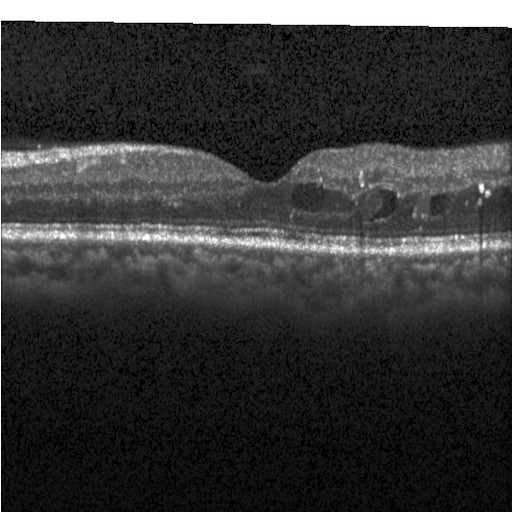

Retinal OCT cross-section · SD-OCT · Heidelberg Spectralis OCT system.
OCT finding: diabetic macular edema (DME).